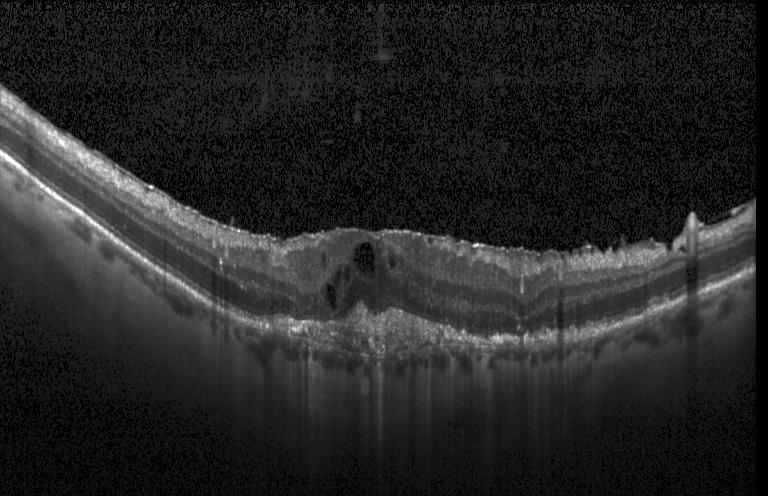 Optical coherence tomography B-scan.
Dx: a choroidal neovascular membrane.